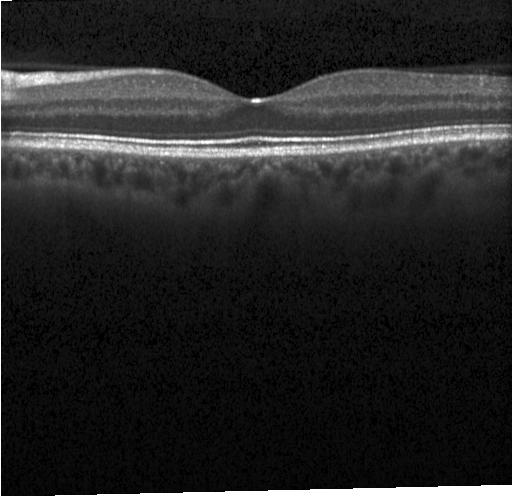
OCT B-scan.
No choroidal neovascularization, diabetic macular edema, or drusen.